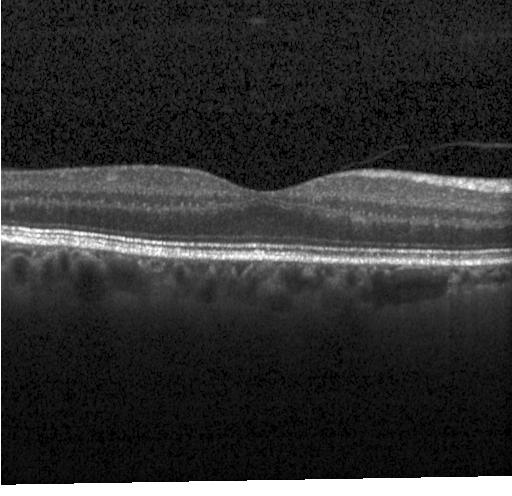

Heidelberg Spectralis, horizontal scan through the fovea, retinal OCT cross-section — Finding: no CNV, DME, or drusen.